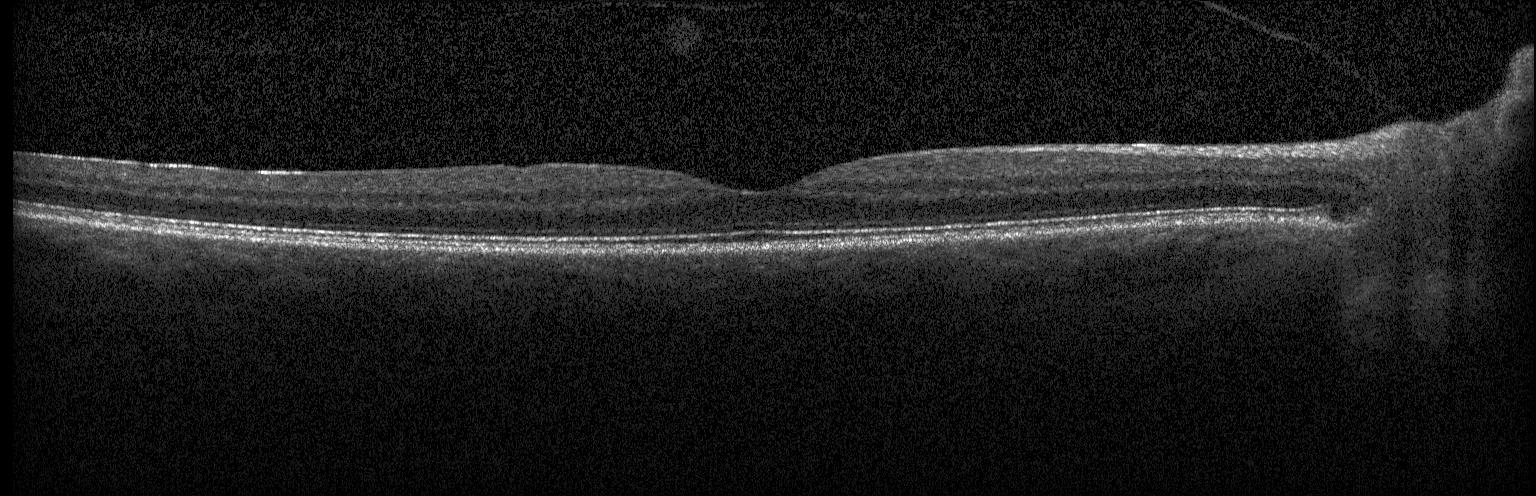

OCT finding: no choroidal neovascularization, no diabetic macular edema, and no drusen.